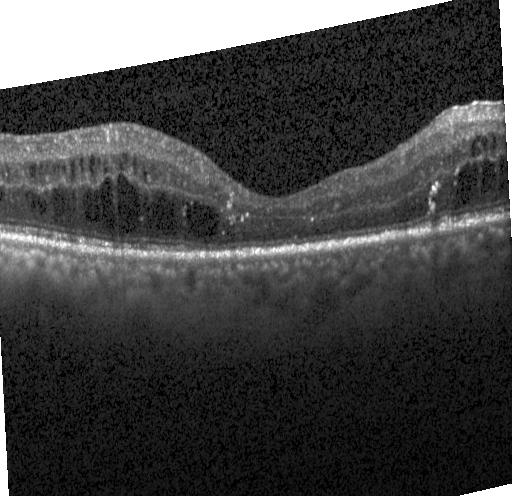
Acquired on a Heidelberg Spectralis · optical coherence tomography B-scan
Impression: diabetic macular edema (DME).